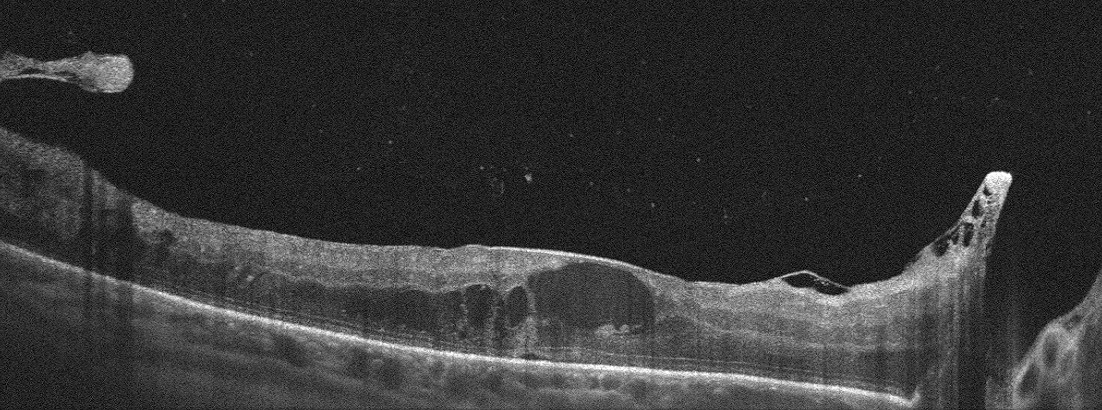

Impression: diabetic macular edema (DME).